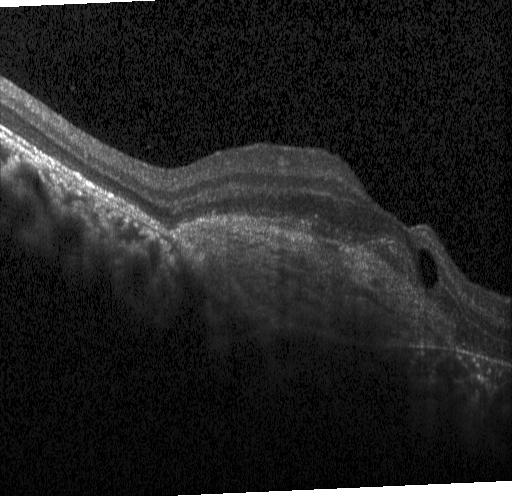

OCT B-scan · macular scan · spectral-domain optical coherence tomography
Diagnosis: choroidal neovascularization (CNV).